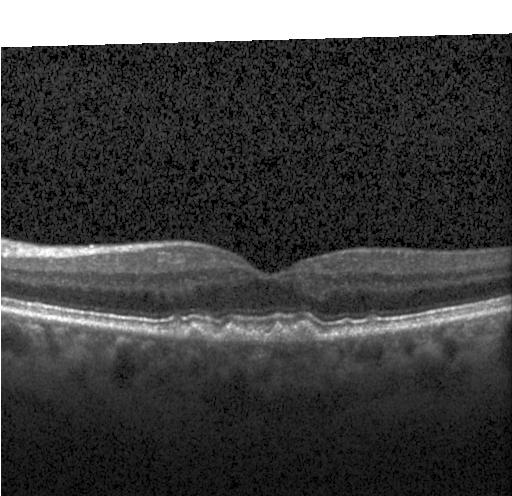 Optical coherence tomography scan. Heidelberg Spectralis OCT system
Drusen.